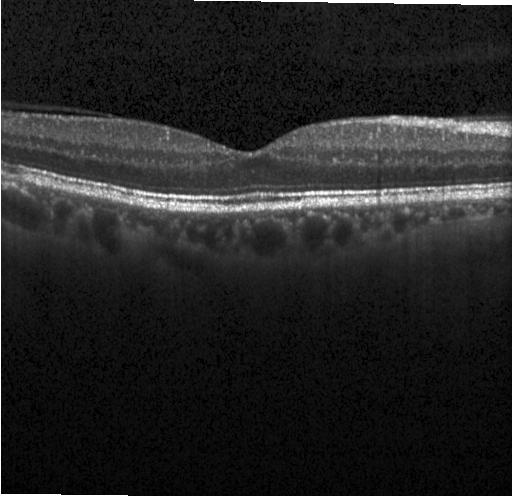 Spectral-domain OCT B-scan: no evidence of choroidal neovascularization, diabetic macular edema, or drusen.